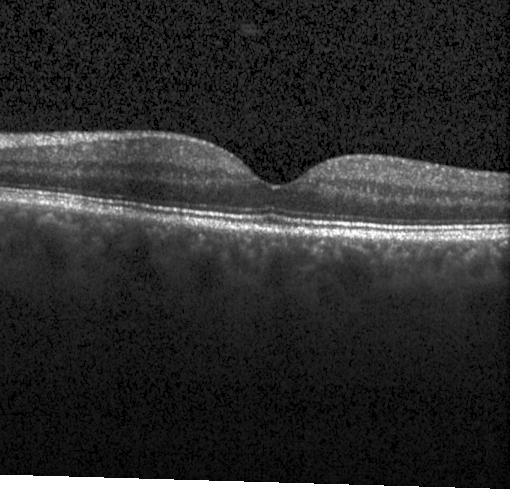 SD-OCT · optical coherence tomography B-scan.
Diagnosis: neither CNV, DME, nor drusen.